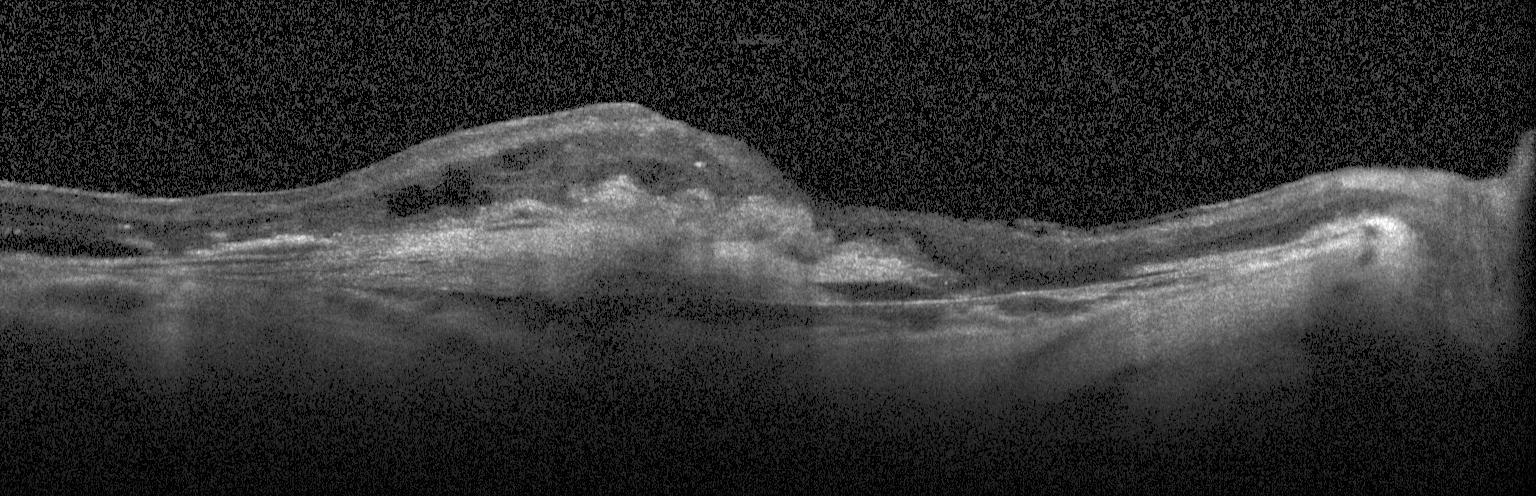 Optical coherence tomography scan
Finding: choroidal neovascularization.